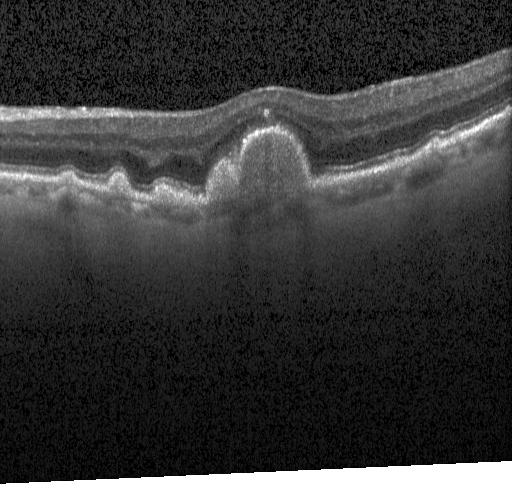

Optical coherence tomography scan.
Diagnosis: drusen.